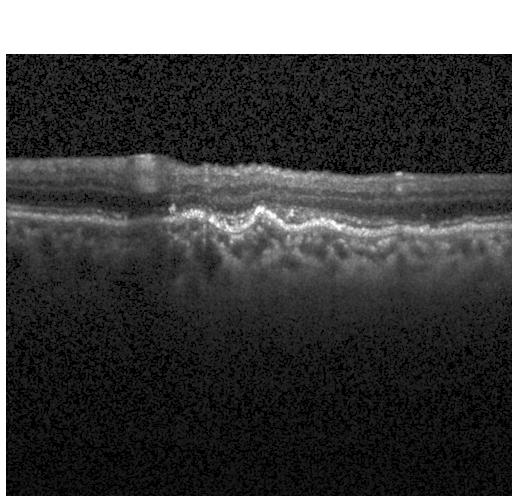 Instrument: Heidelberg Spectralis · SD-OCT · optical coherence tomography scan — Macular OCT: a choroidal neovascular membrane.